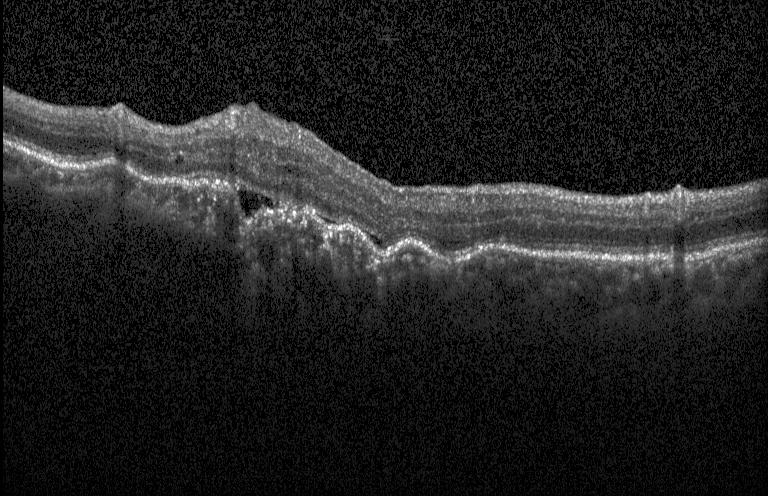 Retinal OCT B-scan, macular scan, acquired on a Heidelberg Spectralis, spectral-domain OCT — Impression: choroidal neovascularization (CNV).